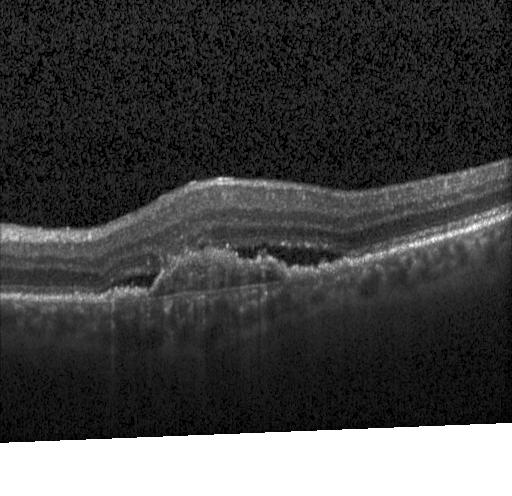

Dx: CNV.